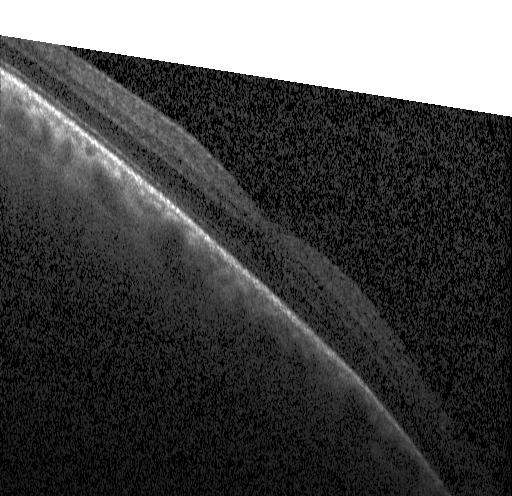
OCT B-scan showing no evidence of CNV, DME, or drusen.